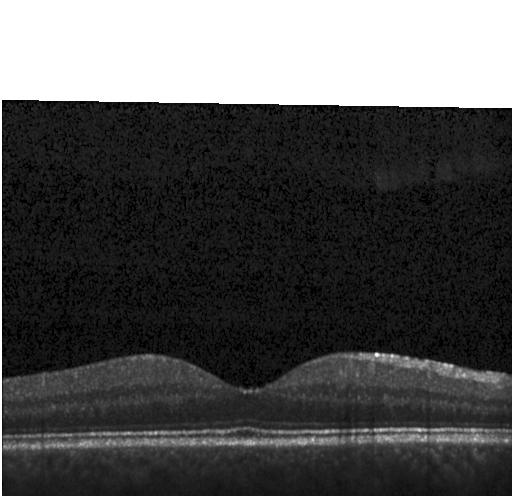
Macular OCT: no choroidal neovascularization, no diabetic macular edema, and no drusen.